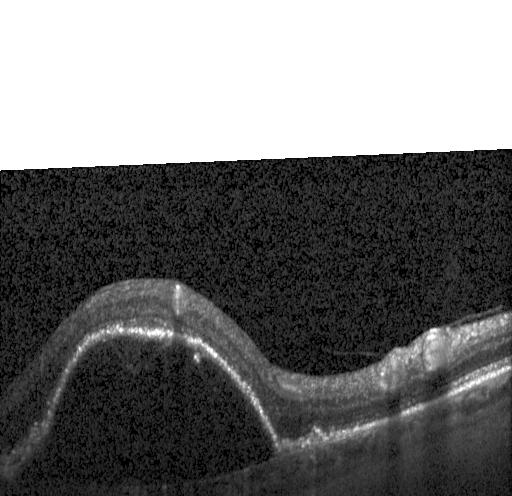 Retinal OCT cross-section showing choroidal neovascularization (CNV).